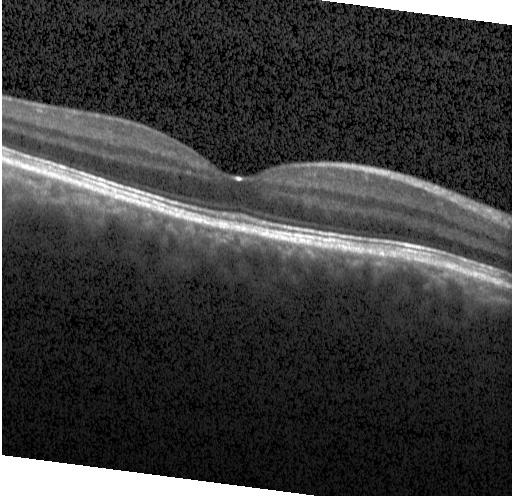 Through the macula · SD-OCT · instrument: Heidelberg Spectralis · OCT line scan
This B-scan demonstrates no choroidal neovascularization, no diabetic macular edema, and no drusen.